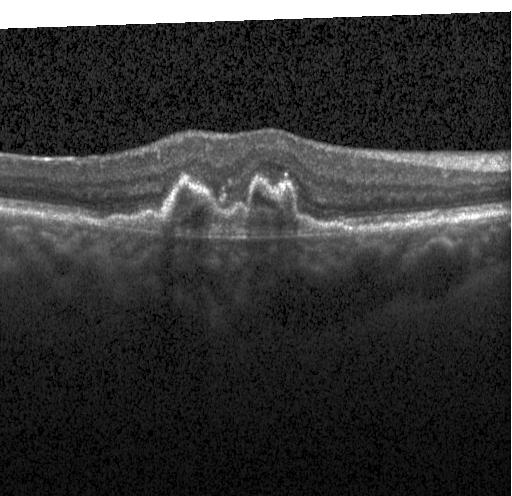
Optical coherence tomography scan. Heidelberg Spectralis OCT system. SD-OCT. Centered on the fovea. A choroidal neovascular membrane.